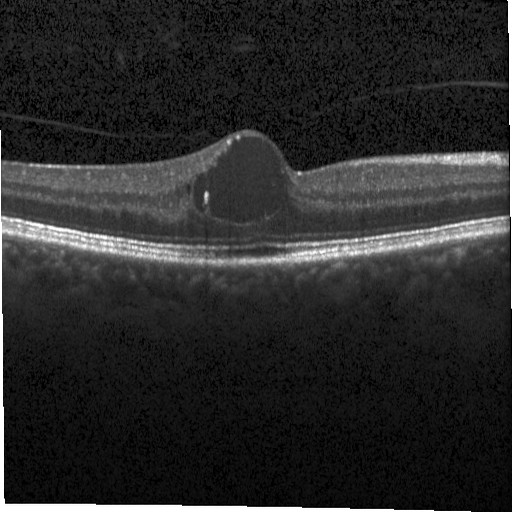 Macular scan; OCT line scan; spectral-domain optical coherence tomography. Finding: diabetic macular edema (DME).